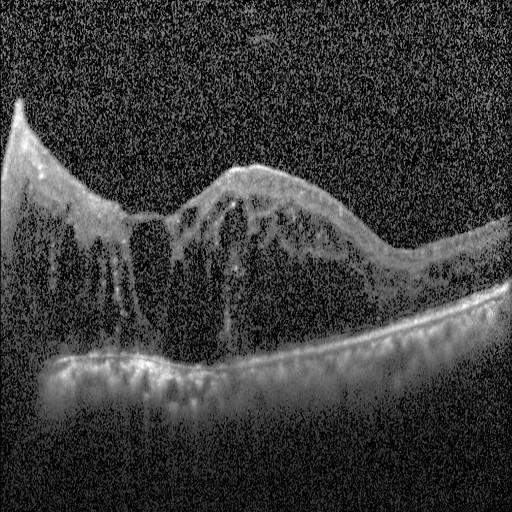

Macular OCT demonstrating DME.